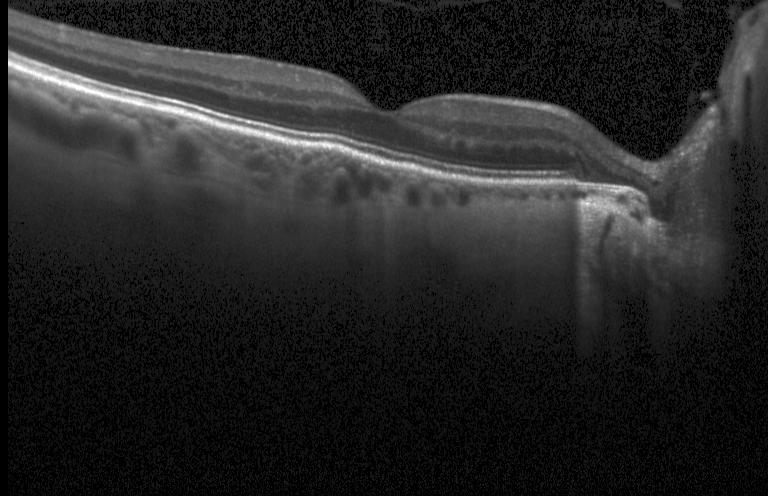 Assessment: neither choroidal neovascularization, diabetic macular edema, nor drusen.